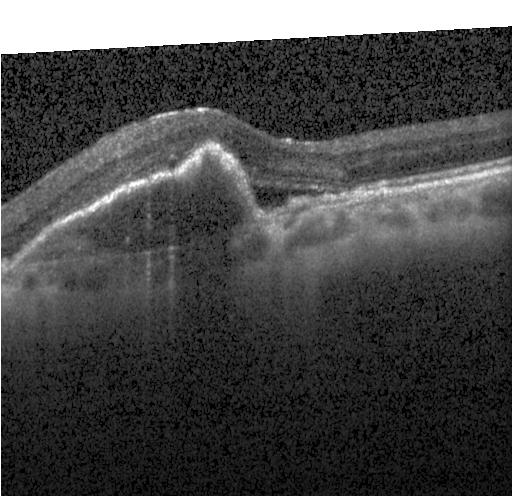 Through the macula · retinal OCT B-scan · acquired on a Heidelberg Spectralis
Macular OCT: CNV.